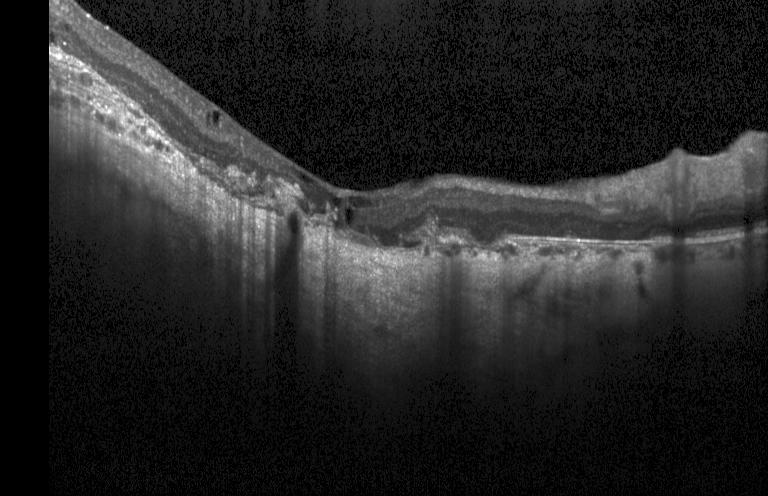
Dx: choroidal neovascularization (CNV).